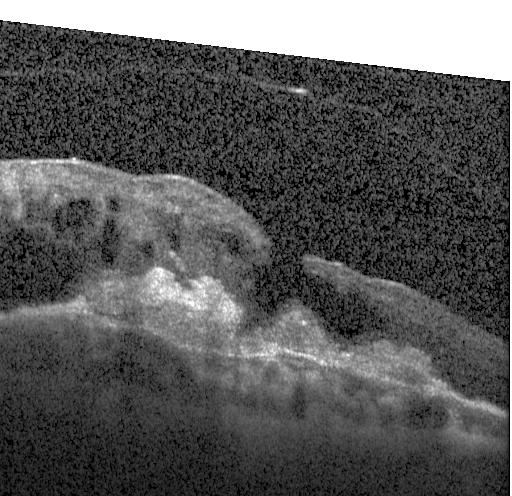

Optical coherence tomography scan. Spectral-domain optical coherence tomography. Centered on the fovea. Assessment: CNV.